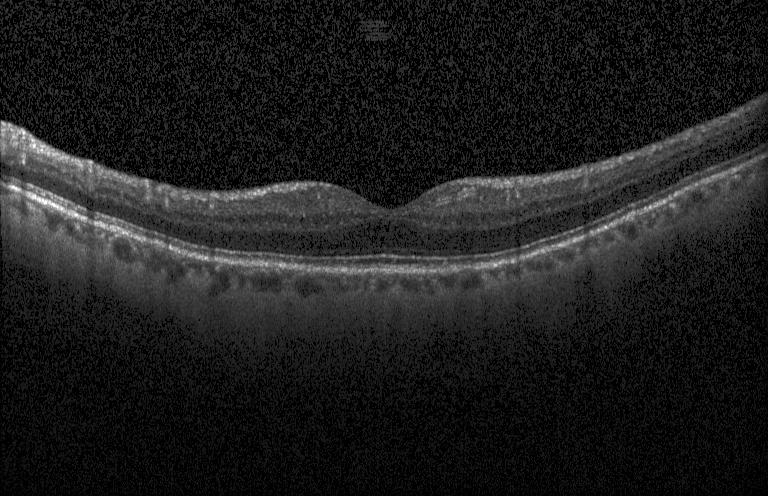
Acquired on a Heidelberg Spectralis, spectral-domain OCT, optical coherence tomography scan, fovea-centered.
The scan shows no evidence of CNV, DME, or drusen.